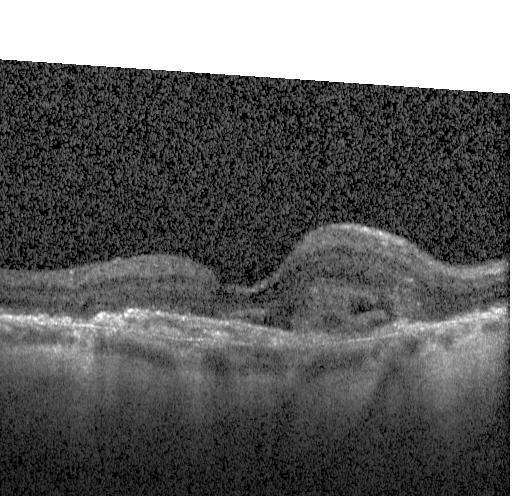

OCT line scan
OCT finding: a choroidal neovascular membrane.